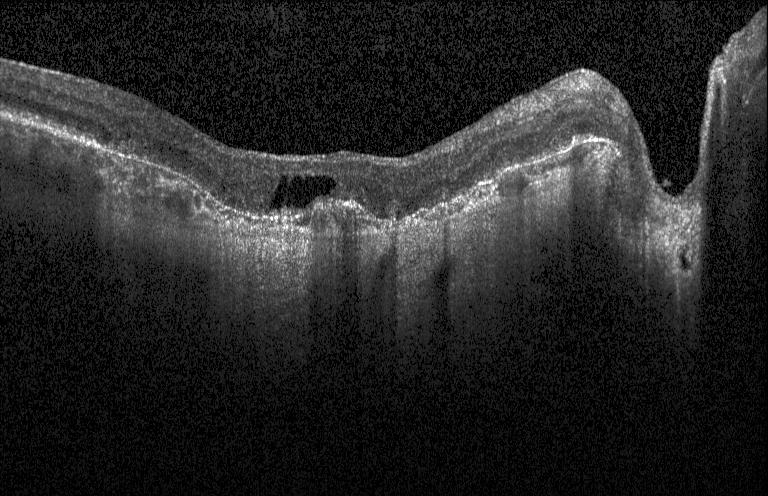

Retinal OCT B-scan · fovea-centered · SD-OCT.
Macular OCT: choroidal neovascularization.